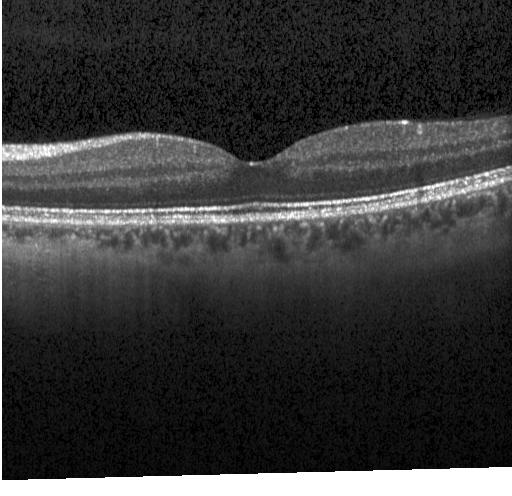

Optical coherence tomography scan. SD-OCT. Centered on the fovea. Acquired on a Heidelberg Spectralis.
Diagnosis: neither choroidal neovascularization, diabetic macular edema, nor drusen.